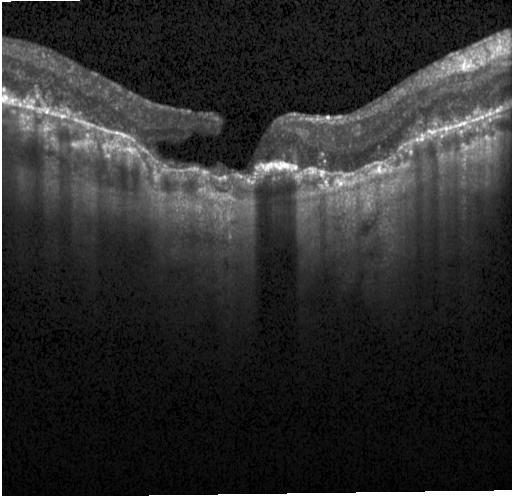
SD-OCT; Heidelberg Spectralis; centered on the fovea; retinal OCT B-scan
Impression: a choroidal neovascular membrane.